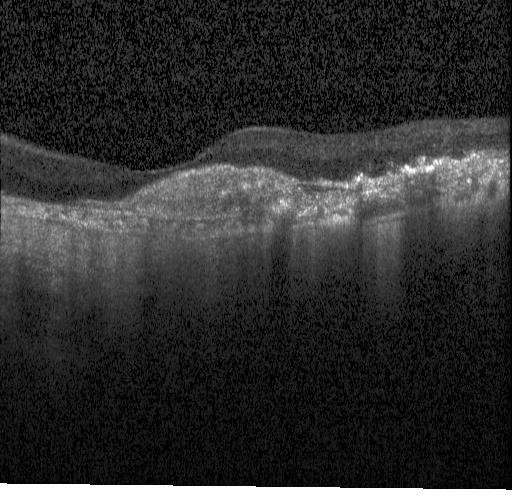
Spectral-domain OCT · centered on the fovea · optical coherence tomography B-scan.
OCT finding: a choroidal neovascular membrane.